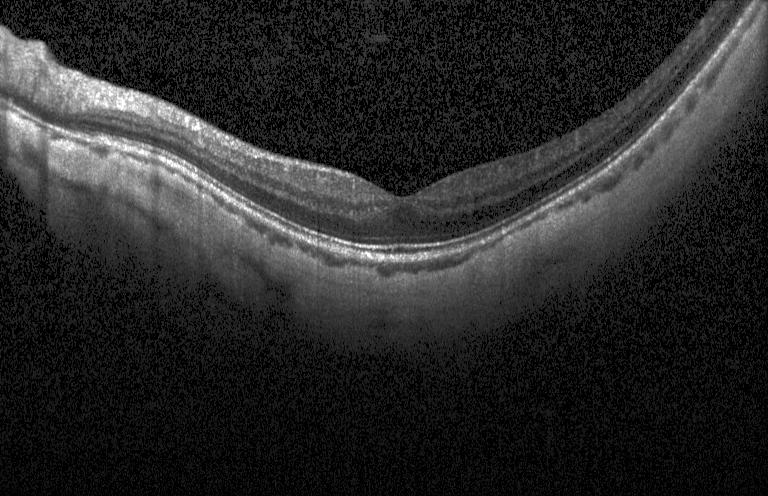 OCT line scan — Impression: neither choroidal neovascularization, diabetic macular edema, nor drusen.